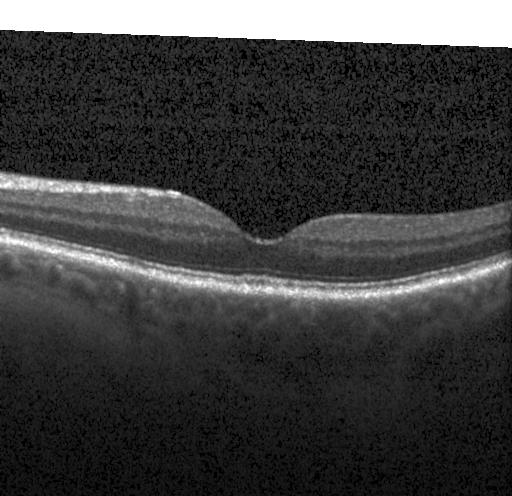
OCT B-scan. Finding: neither choroidal neovascularization, diabetic macular edema, nor drusen.